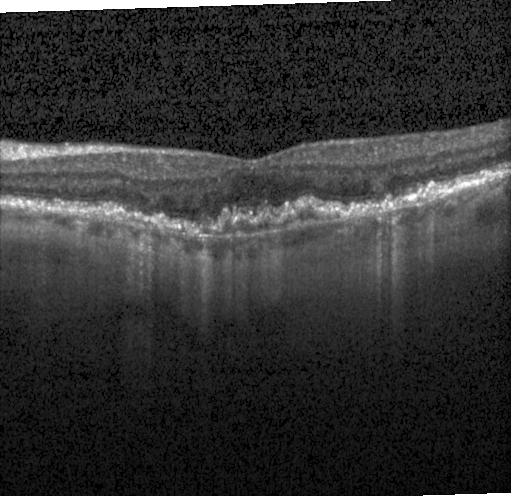 OCT finding: a choroidal neovascular membrane.